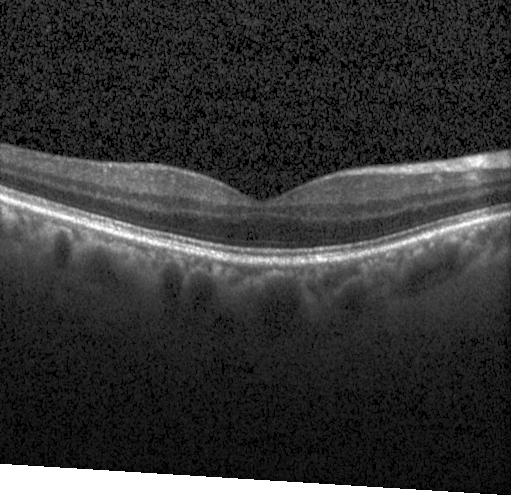 Fovea-centered, retinal OCT B-scan. Dx: no choroidal neovascularization, diabetic macular edema, or drusen.